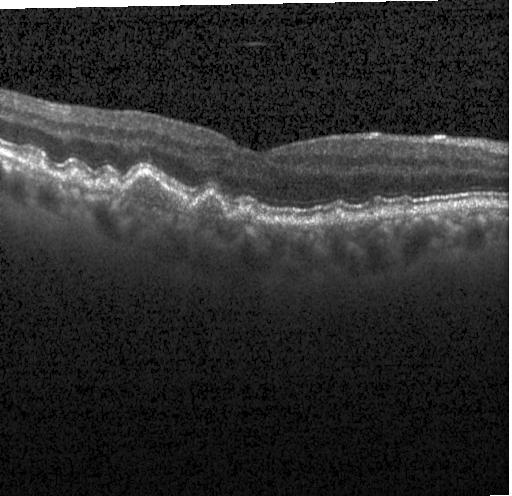

Spectral-domain OCT B-scan: drusen.